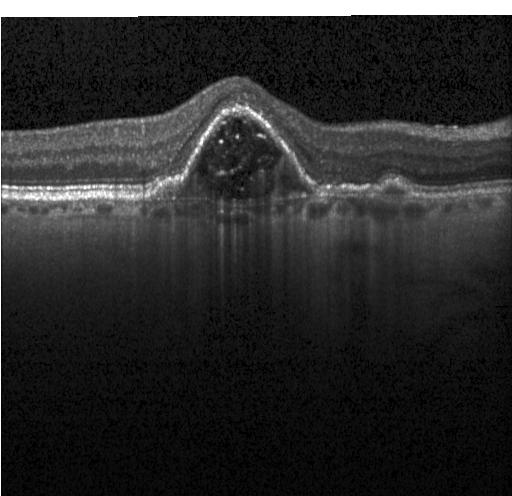 OCT B-scan
Finding: choroidal neovascularization.